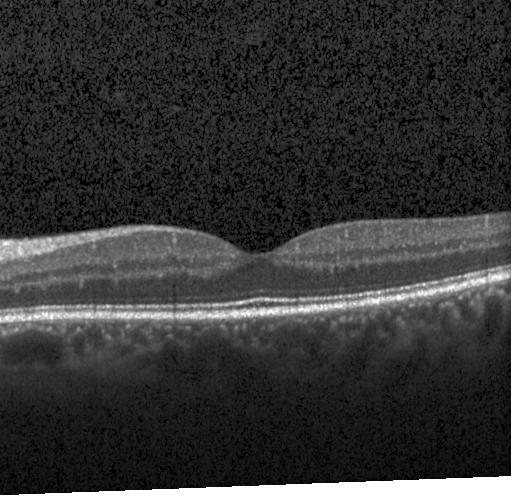 Finding: no evidence of CNV, DME, or drusen.